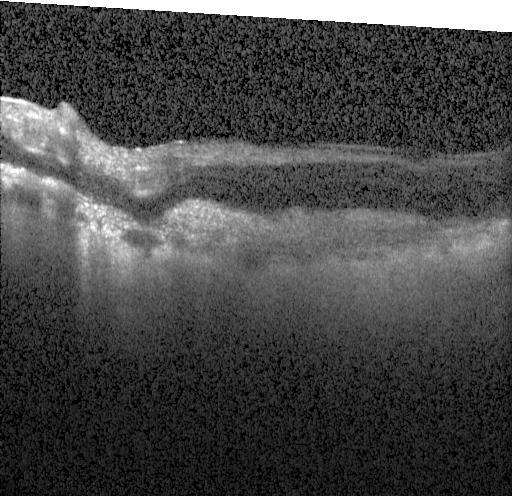 Impression: a choroidal neovascular membrane.